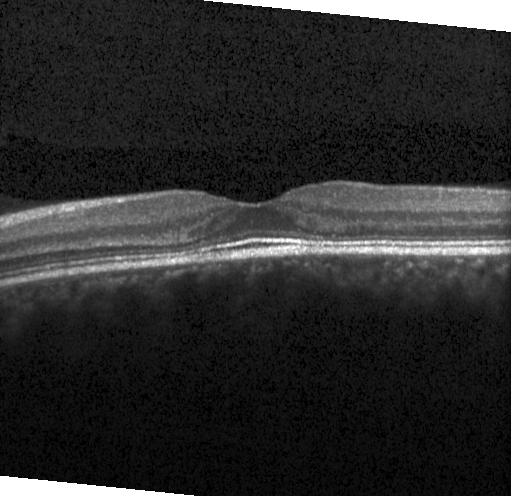
The scan shows neither choroidal neovascularization, diabetic macular edema, nor drusen.